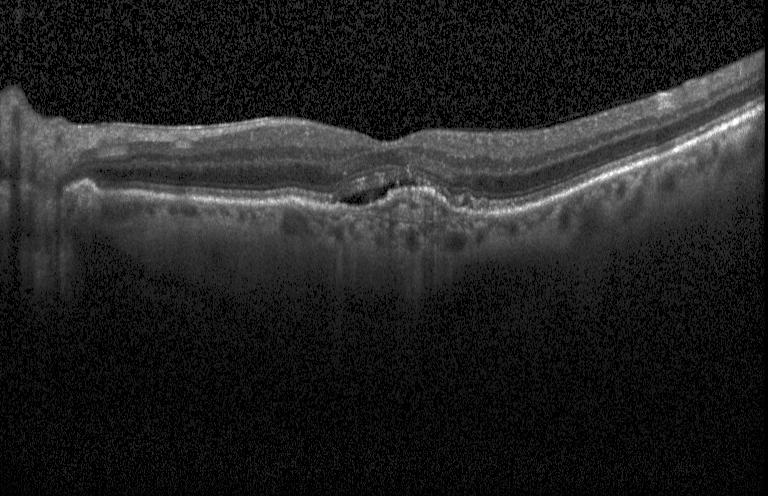 OCT B-scan; spectral-domain OCT; instrument: Heidelberg Spectralis. Dx: CNV.